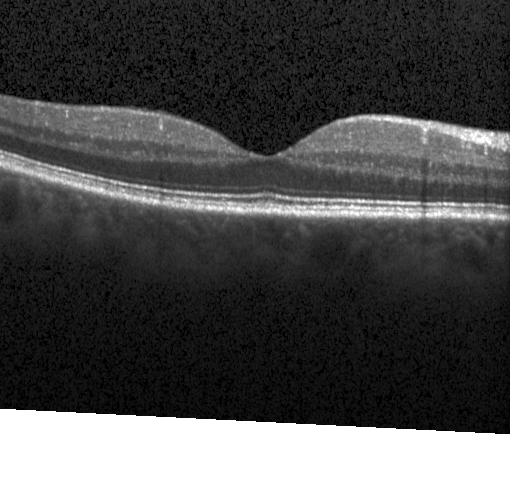

This B-scan demonstrates no choroidal neovascularization, no diabetic macular edema, and no drusen.